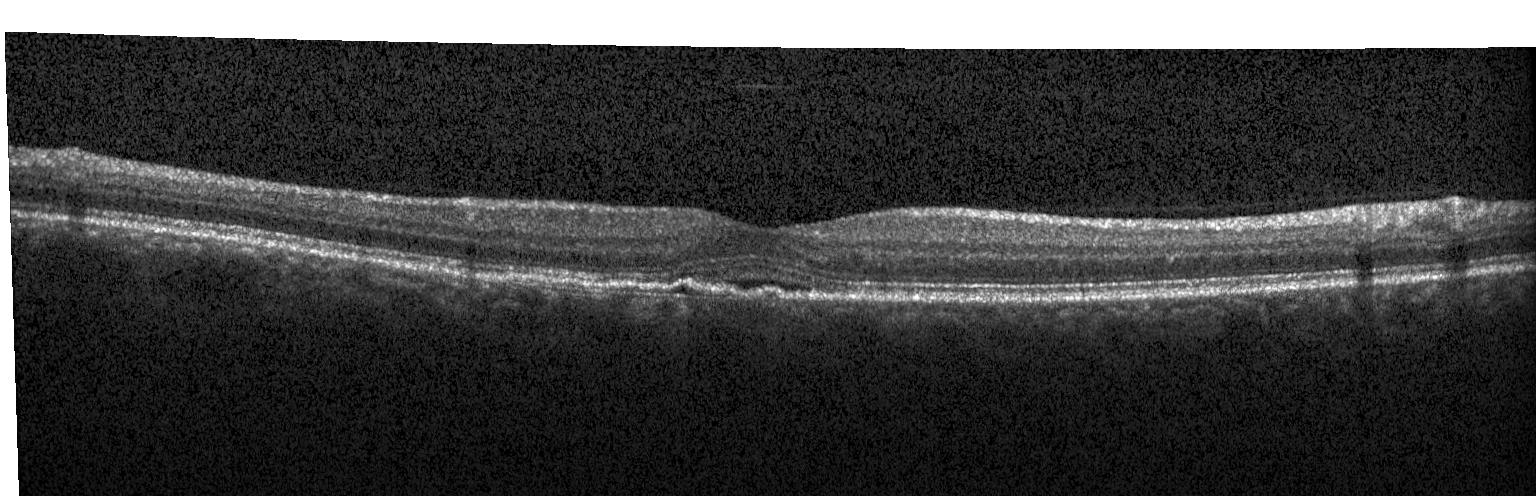

Dx: a choroidal neovascular membrane.